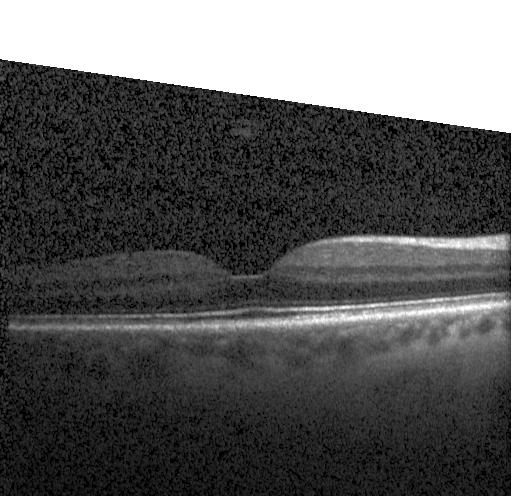
OCT B-scan — Macular OCT: no choroidal neovascularization, diabetic macular edema, or drusen.